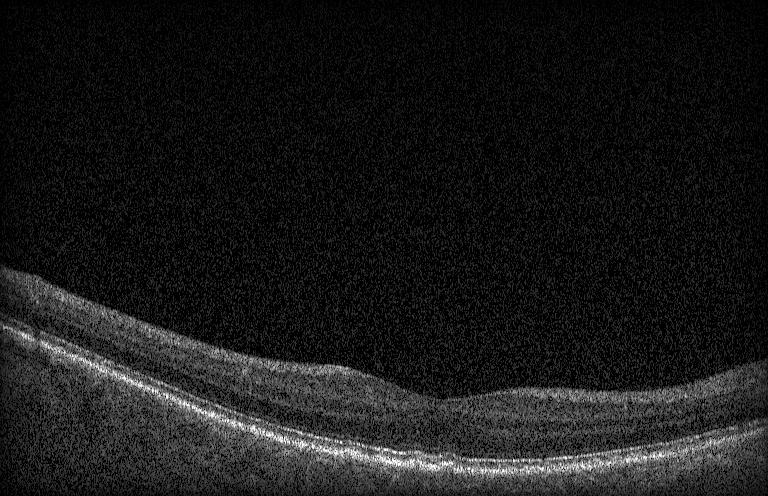
Spectral-domain optical coherence tomography · retinal OCT cross-section · instrument: Heidelberg Spectralis · fovea-centered
The scan shows drusen.